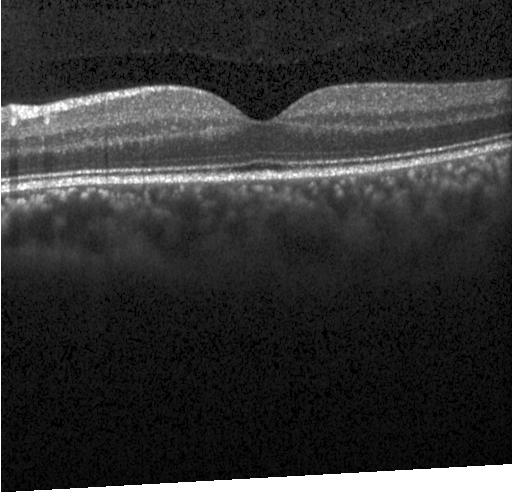

Spectral-domain OCT B-scan: neither choroidal neovascularization, diabetic macular edema, nor drusen.